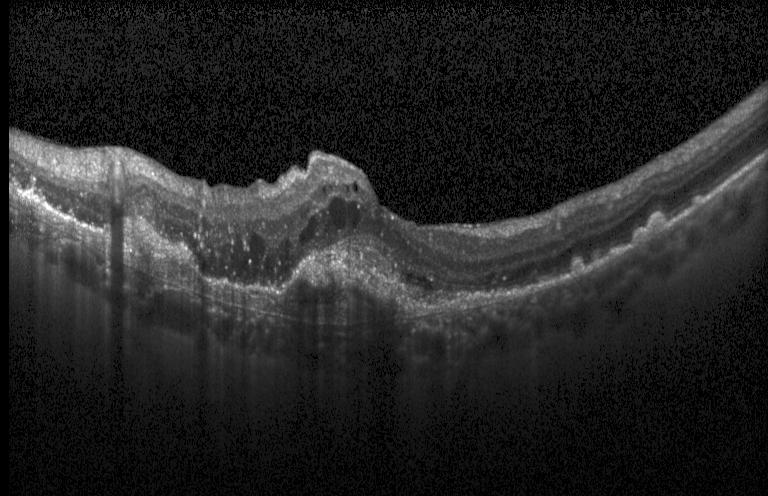

Optical coherence tomography B-scan · spectral-domain OCT — Impression: choroidal neovascularization.